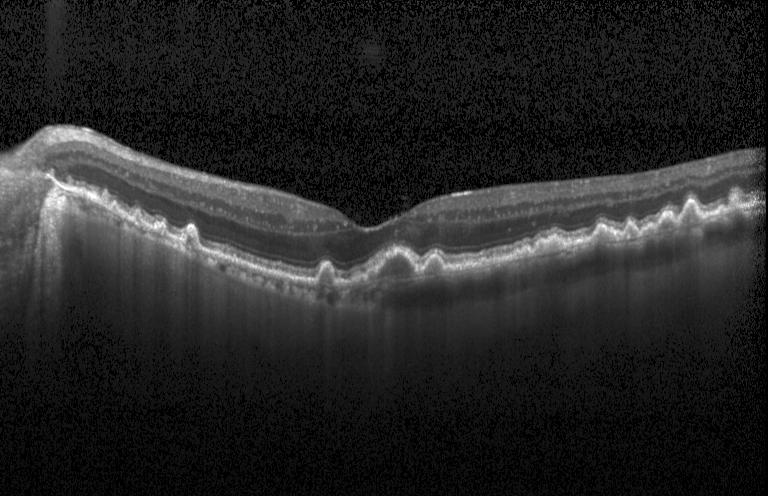
Instrument: Heidelberg Spectralis. Spectral-domain optical coherence tomography. Optical coherence tomography scan — This B-scan demonstrates sub-RPE drusenoid deposits.